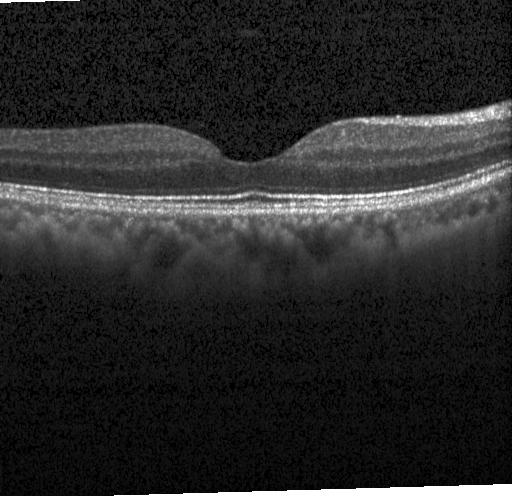 Retinal OCT cross-section
Impression: neither choroidal neovascularization, diabetic macular edema, nor drusen.